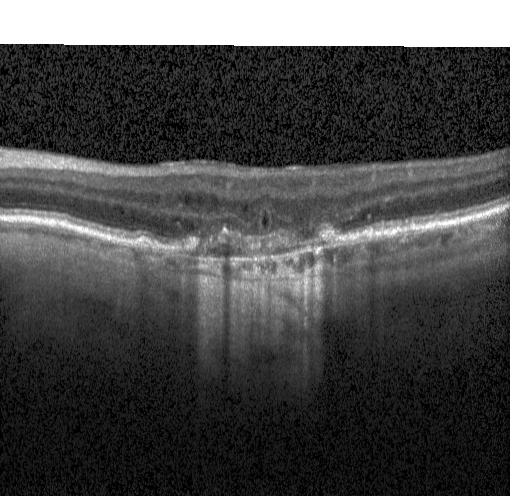
Horizontal scan through the fovea, OCT line scan, Heidelberg Spectralis OCT system.
The scan shows a choroidal neovascular membrane.